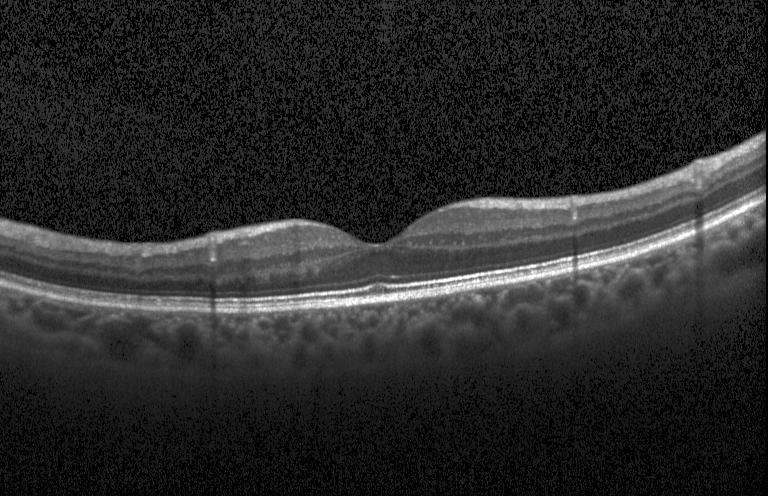
This B-scan demonstrates neither choroidal neovascularization, diabetic macular edema, nor drusen.